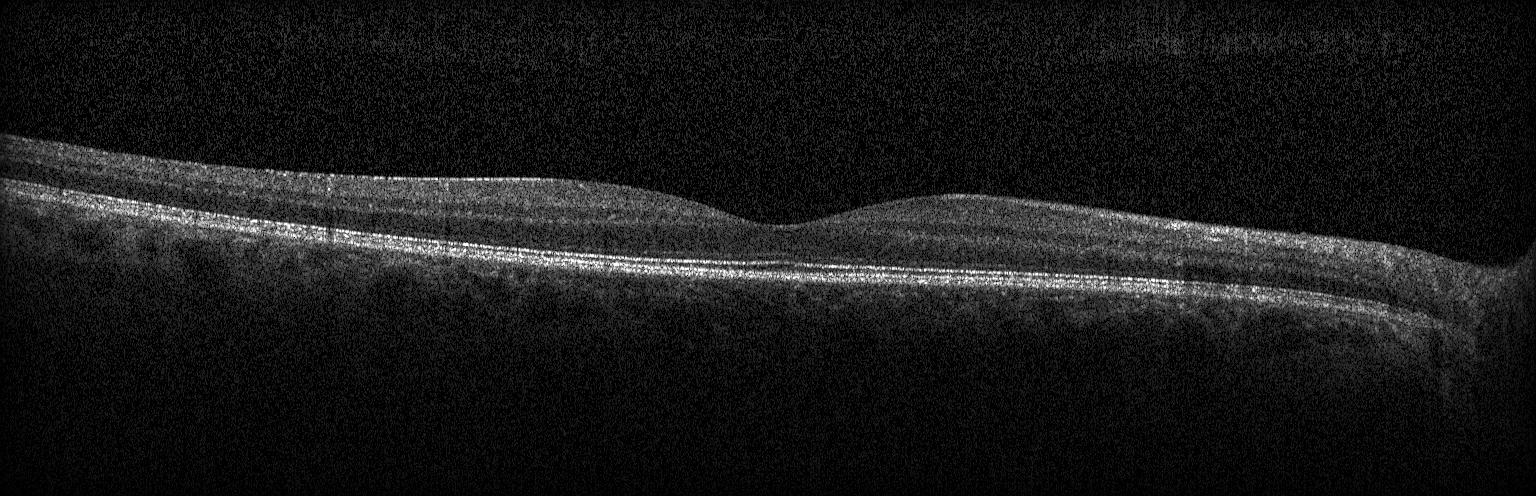

Retinal OCT cross-section · spectral-domain optical coherence tomography
OCT finding: no CNV, DME, or drusen.